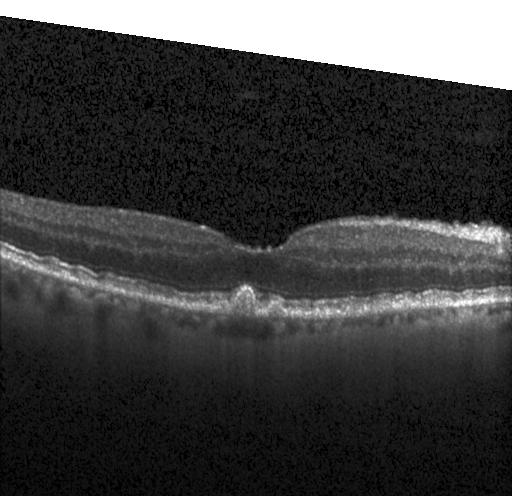 OCT B-scan
Multiple drusen.